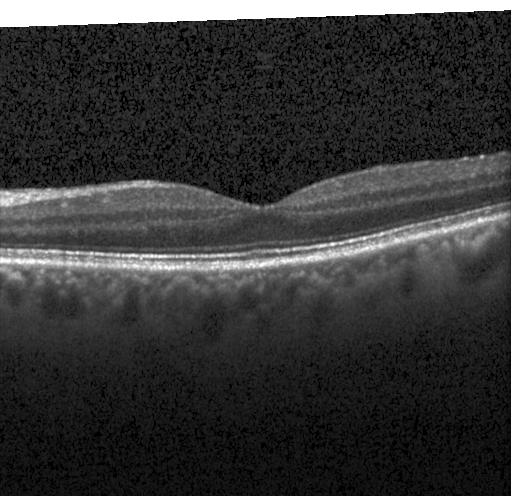

Heidelberg Spectralis · spectral-domain OCT · OCT line scan.
OCT finding: no evidence of choroidal neovascularization, diabetic macular edema, or drusen.